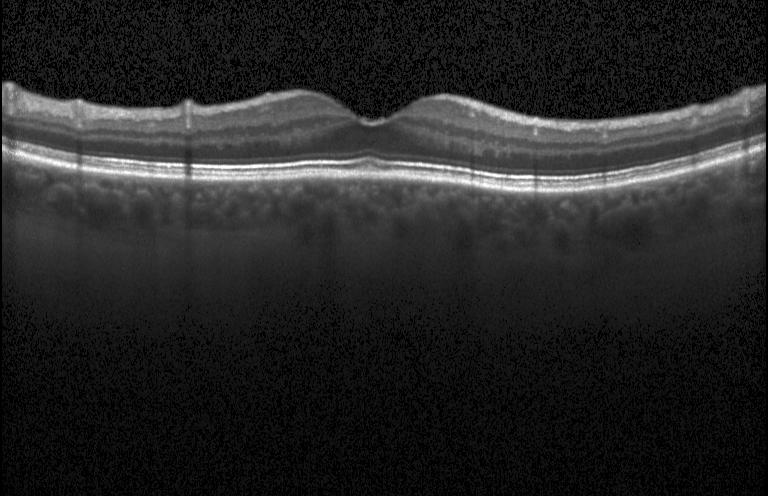

The scan shows no CNV, no DME, and no drusen.